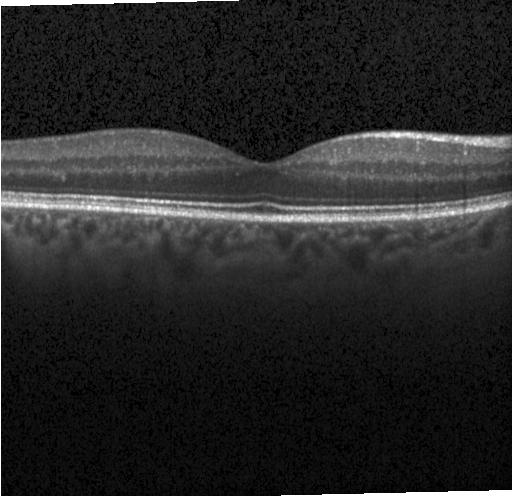
Finding: no choroidal neovascularization, no diabetic macular edema, and no drusen.